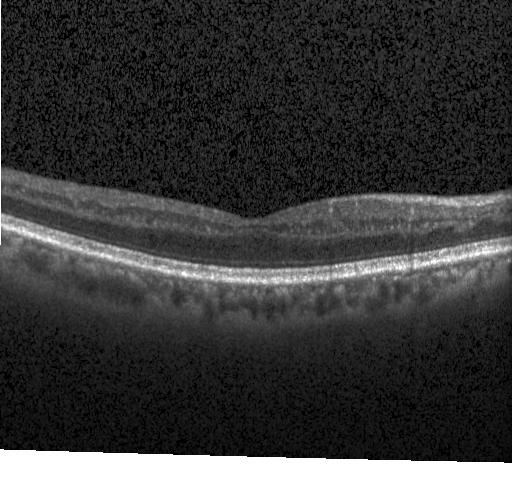
No choroidal neovascularization, diabetic macular edema, or drusen.